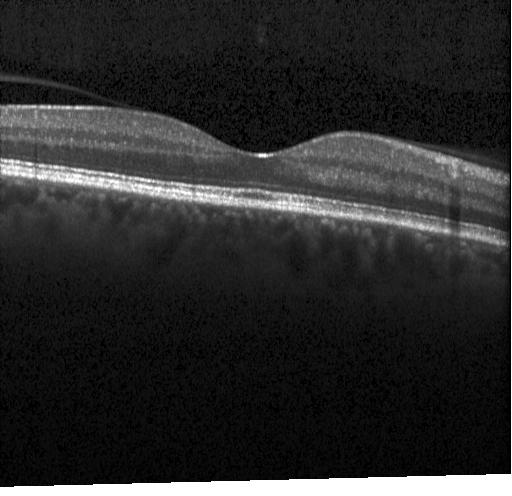
OCT line scan. No CNV, no DME, and no drusen.